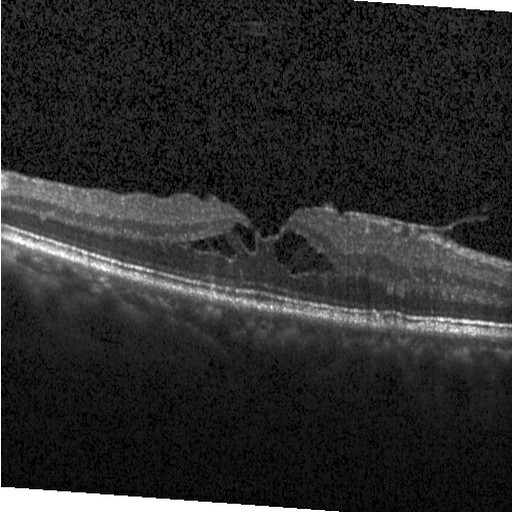

Dx: DME.